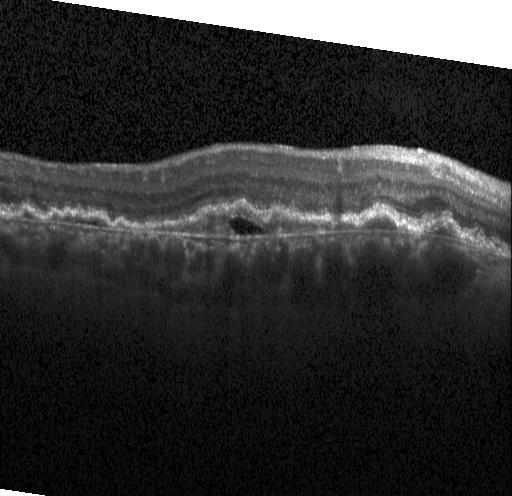

Retinal OCT B-scan.
OCT finding: choroidal neovascularization.